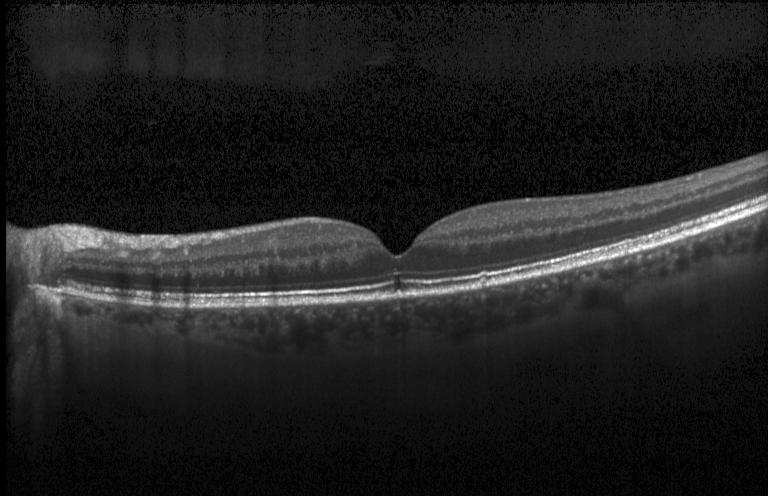
Retinal OCT B-scan — Finding: neither choroidal neovascularization, diabetic macular edema, nor drusen.